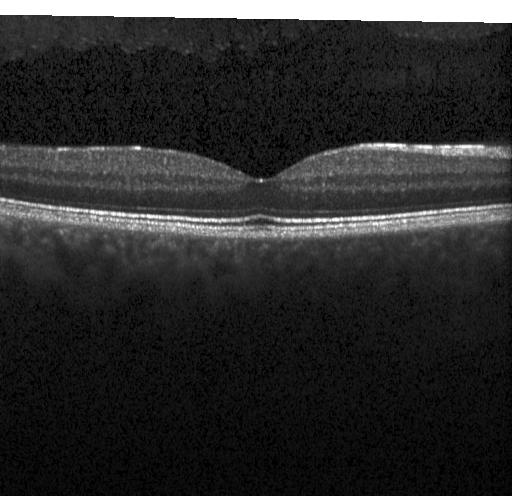

Impression: no choroidal neovascularization, no diabetic macular edema, and no drusen.